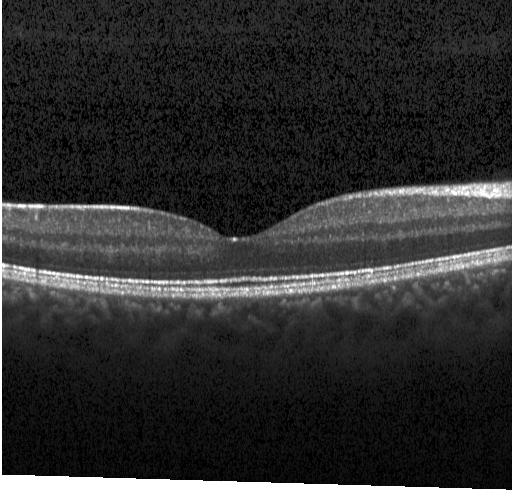
Retinal OCT cross-section · spectral-domain optical coherence tomography · acquired on a Heidelberg Spectralis · fovea-centered
Macular OCT: no evidence of choroidal neovascularization, diabetic macular edema, or drusen.